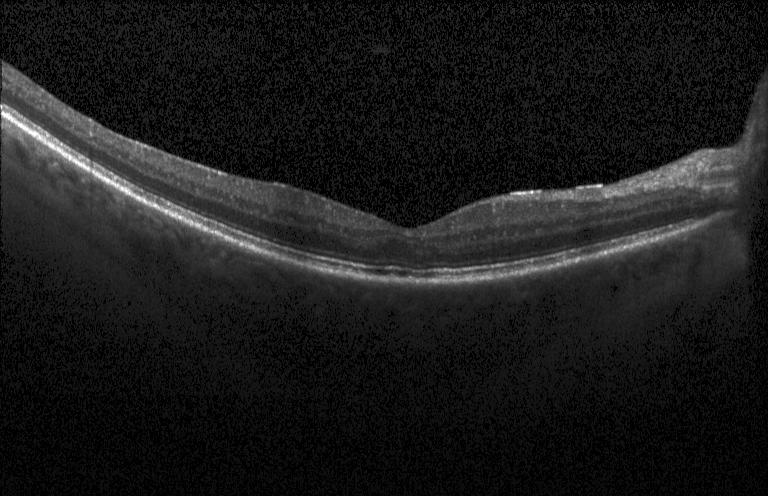 Optical coherence tomography scan. The scan shows no choroidal neovascularization, diabetic macular edema, or drusen.